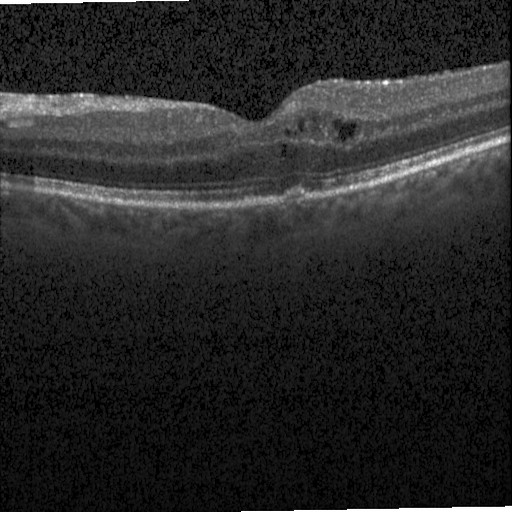
Instrument: Heidelberg Spectralis · fovea-centered · optical coherence tomography B-scan · SD-OCT — Diagnosis: diabetic macular edema (DME).